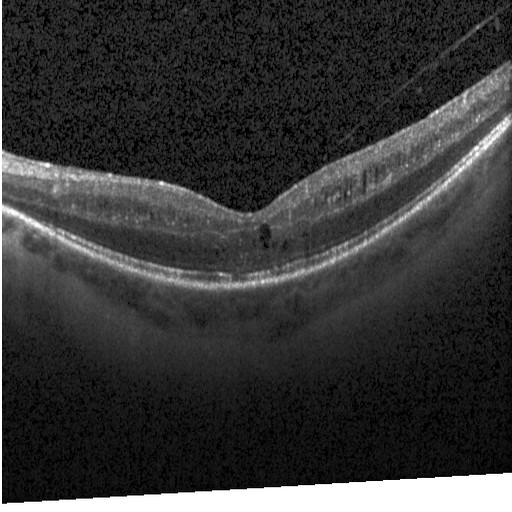

Optical coherence tomography scan.
Impression: diabetic macular edema.